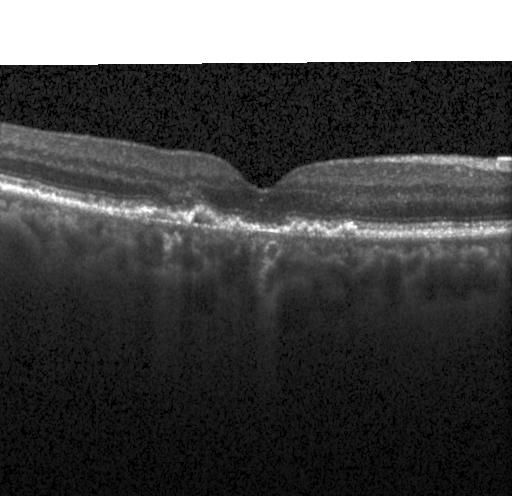 Diagnosis: CNV.